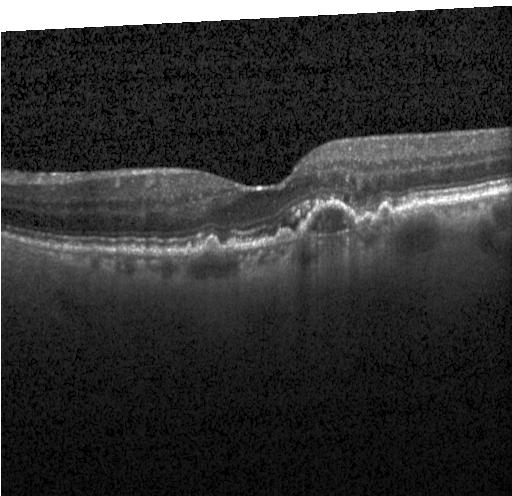 OCT B-scan — Finding: a choroidal neovascular membrane.